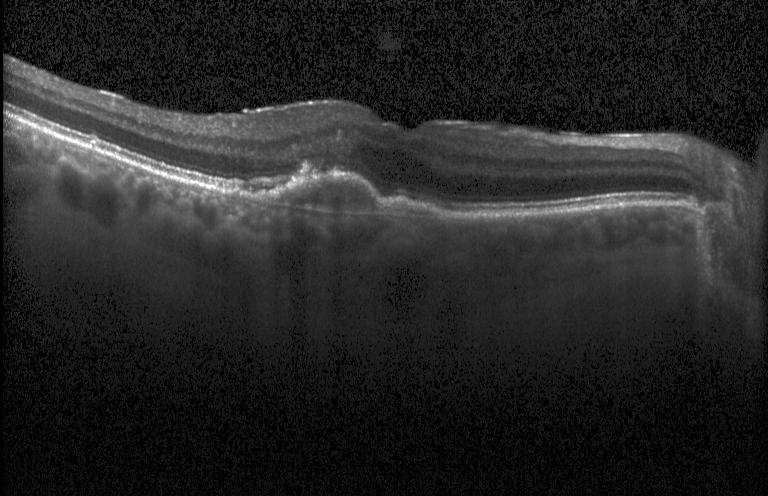
Macular OCT demonstrating choroidal neovascularization.